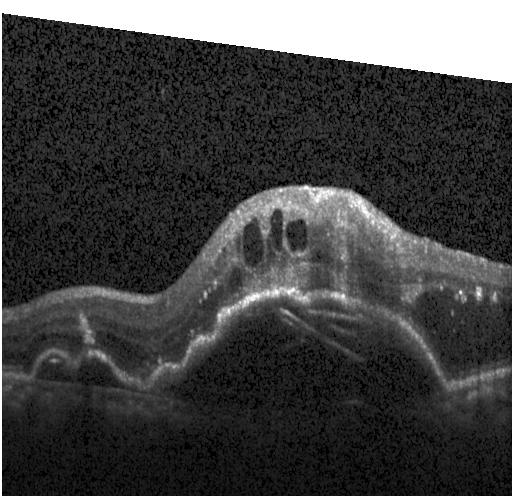

Retinal OCT B-scan
Macular OCT: choroidal neovascularization.